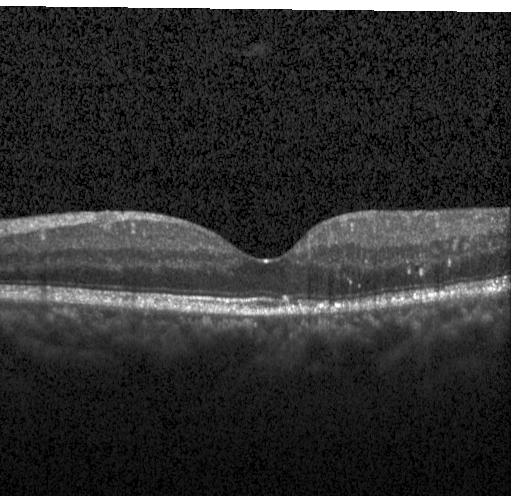
OCT scan showing diabetic macular edema (DME).